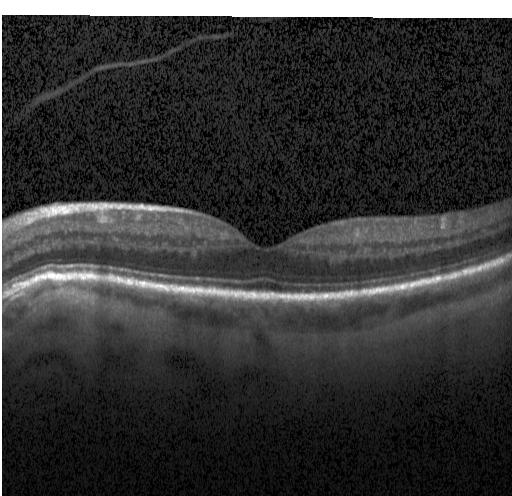

SD-OCT, optical coherence tomography scan, centered on the fovea, acquired on a Heidelberg Spectralis — Finding: neither choroidal neovascularization, diabetic macular edema, nor drusen.